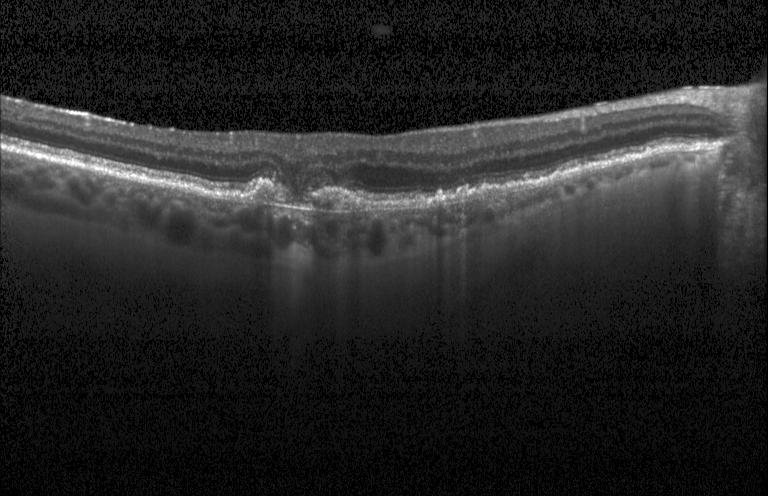
Optical coherence tomography scan
Dx: a choroidal neovascular membrane.